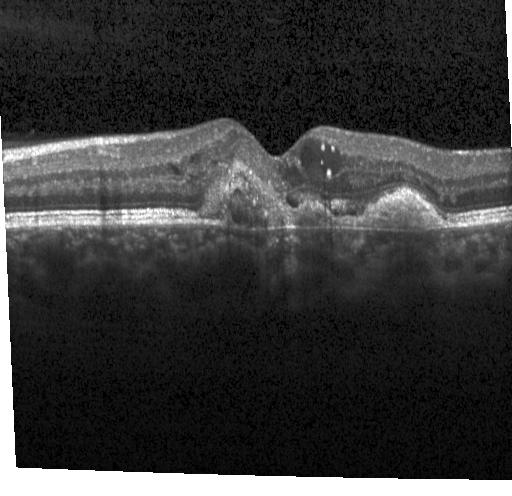 Macular OCT demonstrating choroidal neovascularization.